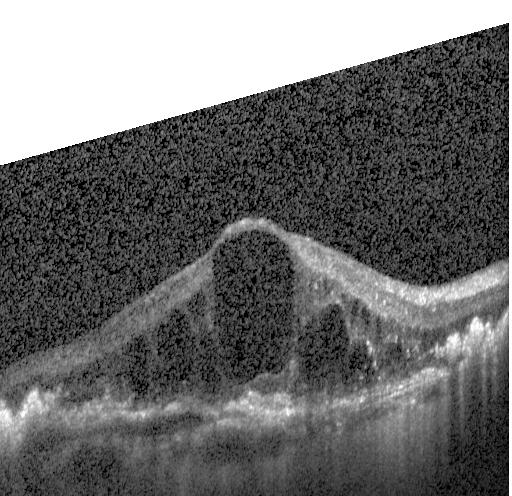 OCT B-scan — Impression: a choroidal neovascular membrane.